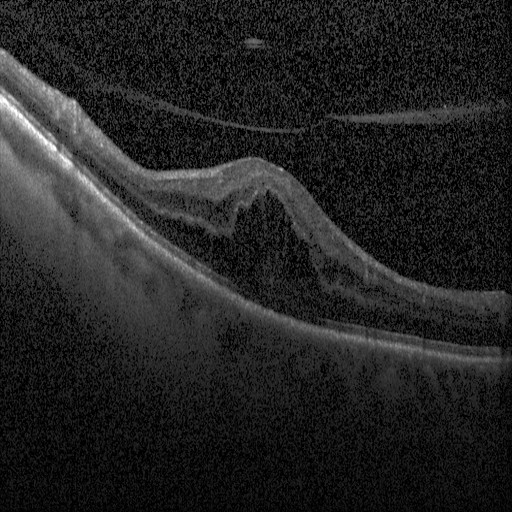 Optical coherence tomography B-scan.
Finding: diabetic macular edema.